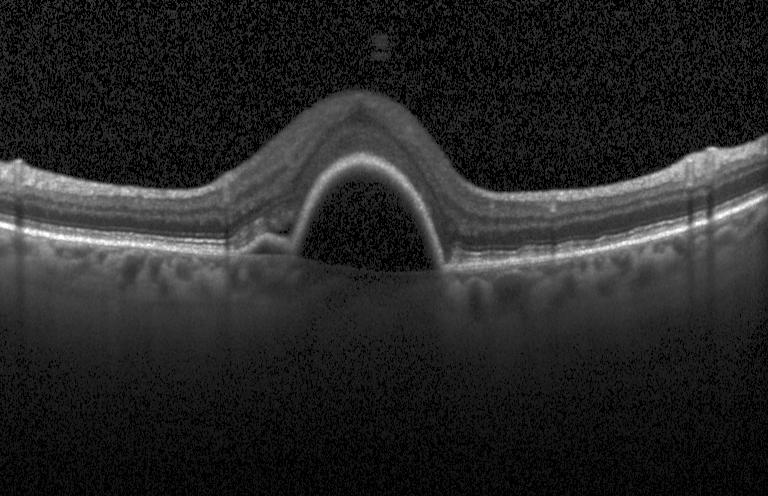
OCT B-scan
Finding: a choroidal neovascular membrane.